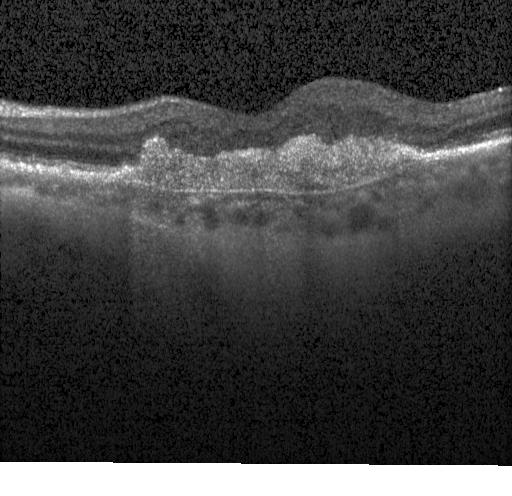 Optical coherence tomography scan · SD-OCT · centered on the fovea · Heidelberg Spectralis OCT system.
Finding: a choroidal neovascular membrane.